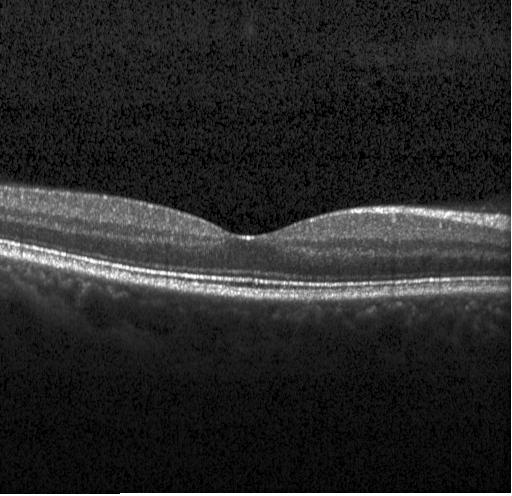
Macular scan; optical coherence tomography scan; Heidelberg Spectralis OCT system; SD-OCT. Macular OCT: no choroidal neovascularization, no diabetic macular edema, and no drusen.